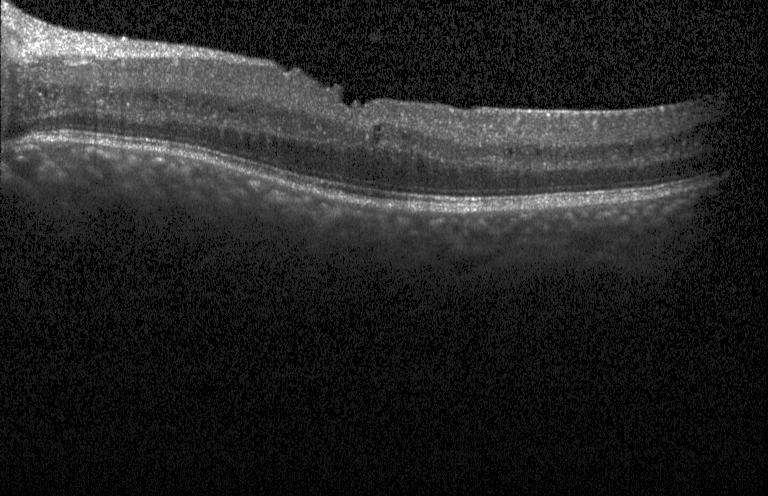 The scan shows diabetic macular edema (DME).